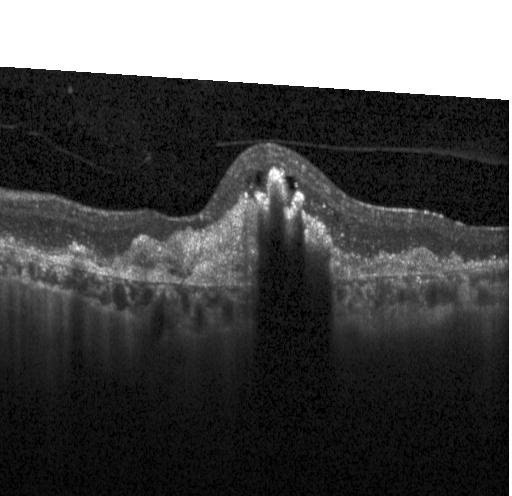

Finding: choroidal neovascularization.